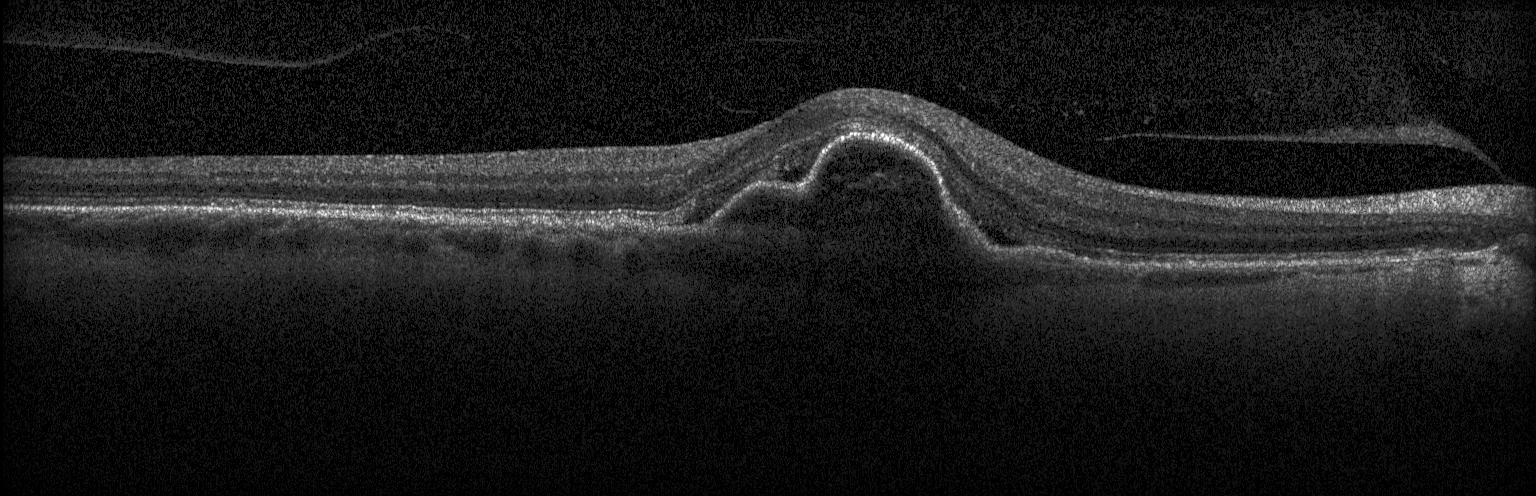

OCT line scan, Heidelberg Spectralis
Finding: choroidal neovascularization (CNV).